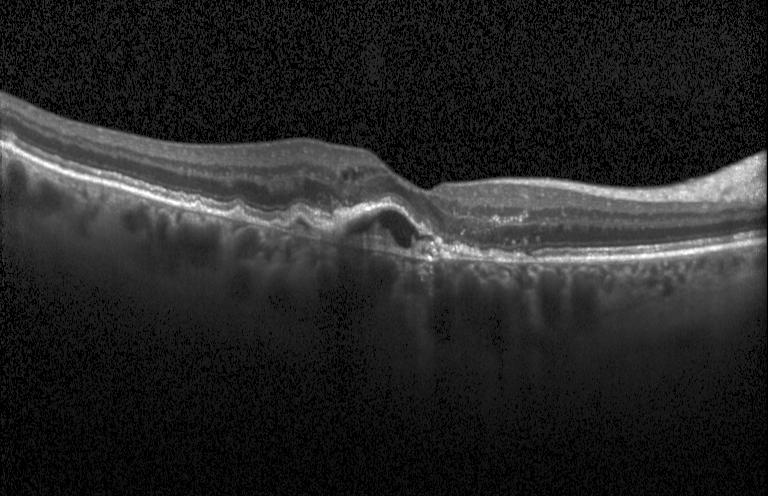 Spectral-domain optical coherence tomography · retinal OCT B-scan · fovea-centered · instrument: Heidelberg Spectralis — Diagnosis: choroidal neovascularization.